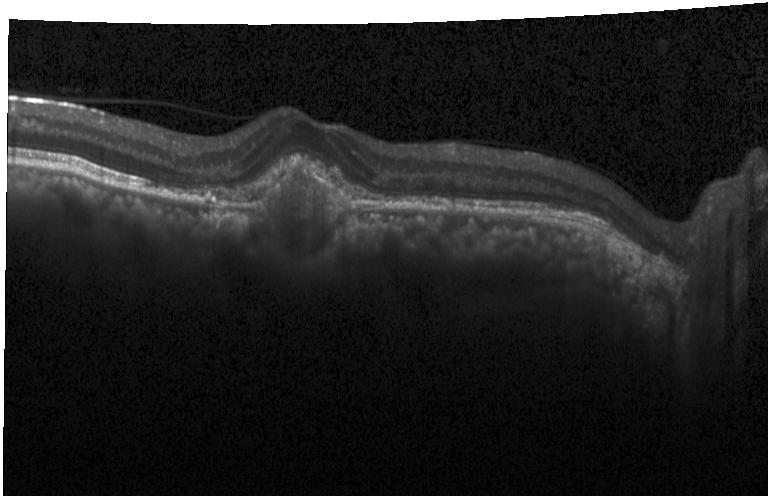 SD-OCT. OCT line scan. Horizontal scan through the fovea.
Dx: choroidal neovascularization.